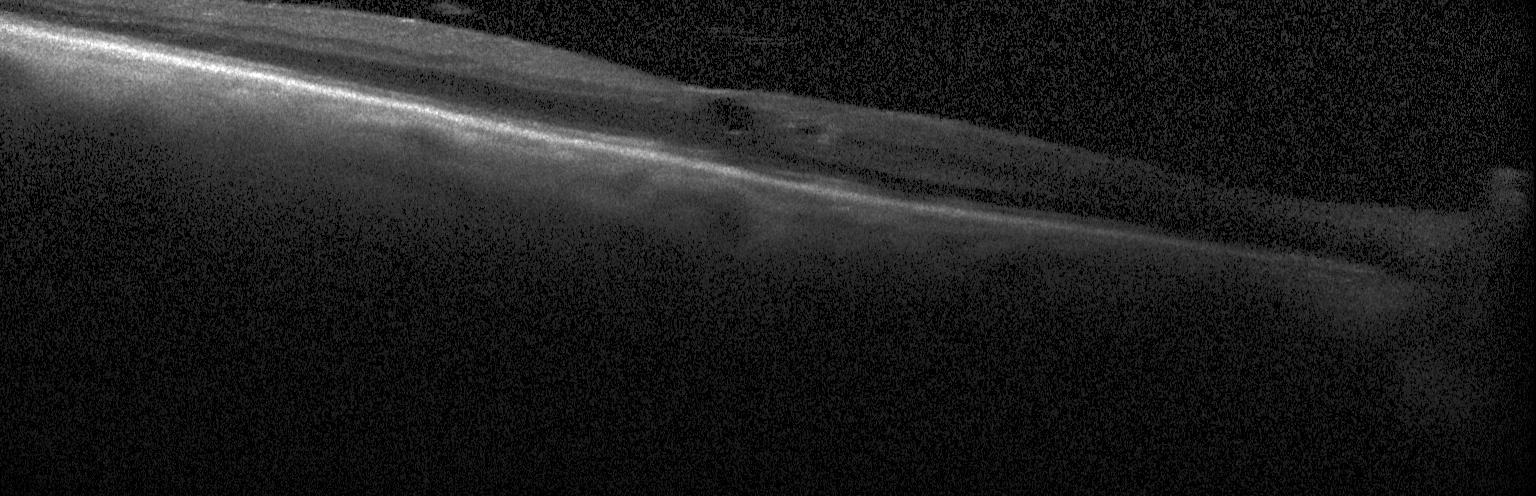 Retinal OCT cross-section · spectral-domain optical coherence tomography · centered on the fovea · instrument: Heidelberg Spectralis — Impression: diabetic macular edema (DME).